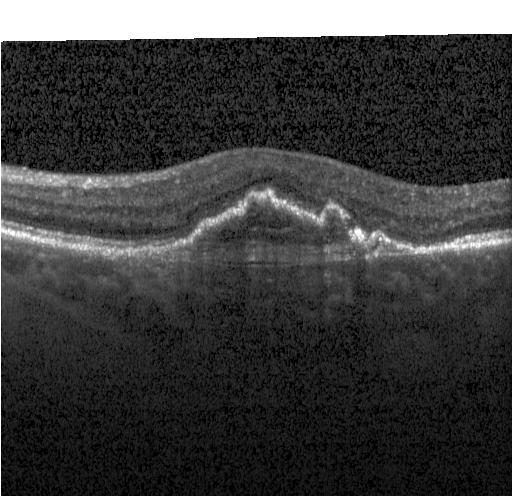

Retinal OCT B-scan.
This B-scan demonstrates choroidal neovascularization.